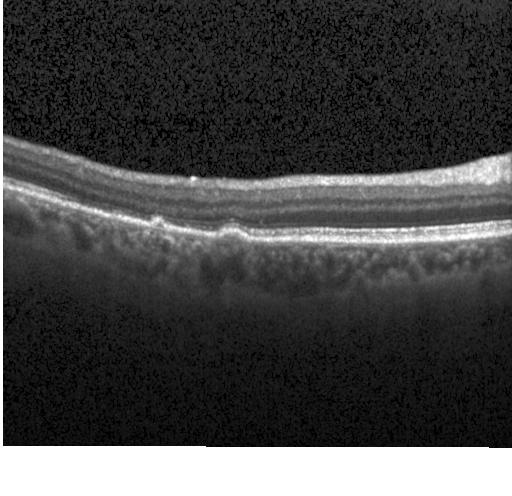
Fovea-centered; acquired on a Heidelberg Spectralis; SD-OCT; optical coherence tomography B-scan. Dx: sub-RPE drusenoid deposits.